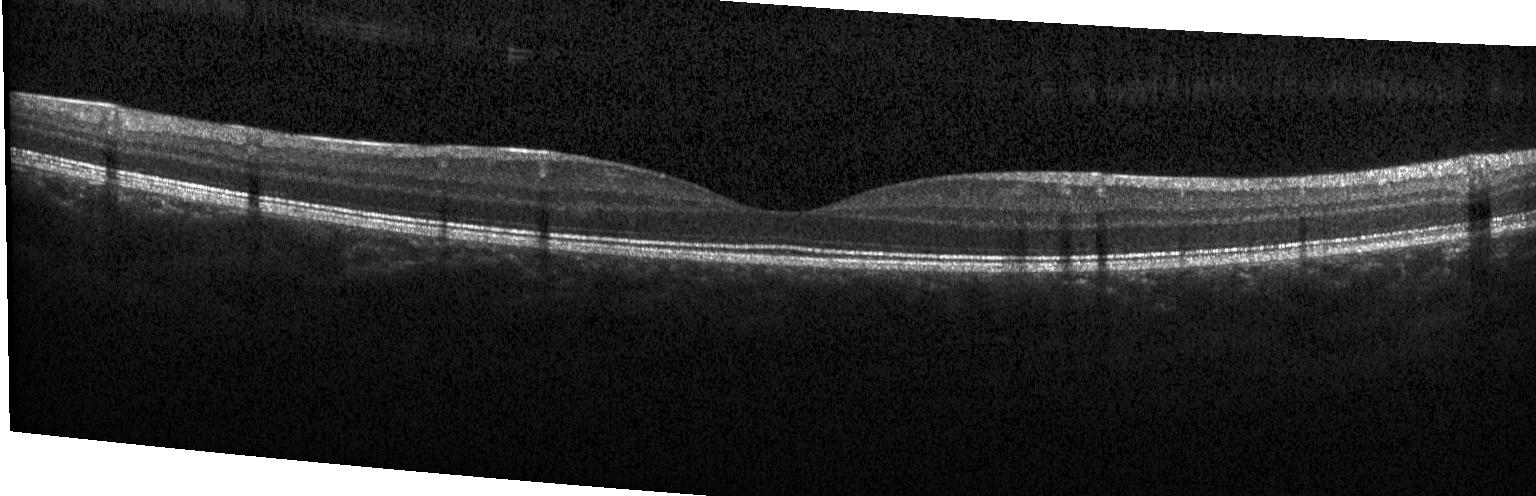 No evidence of choroidal neovascularization, diabetic macular edema, or drusen.